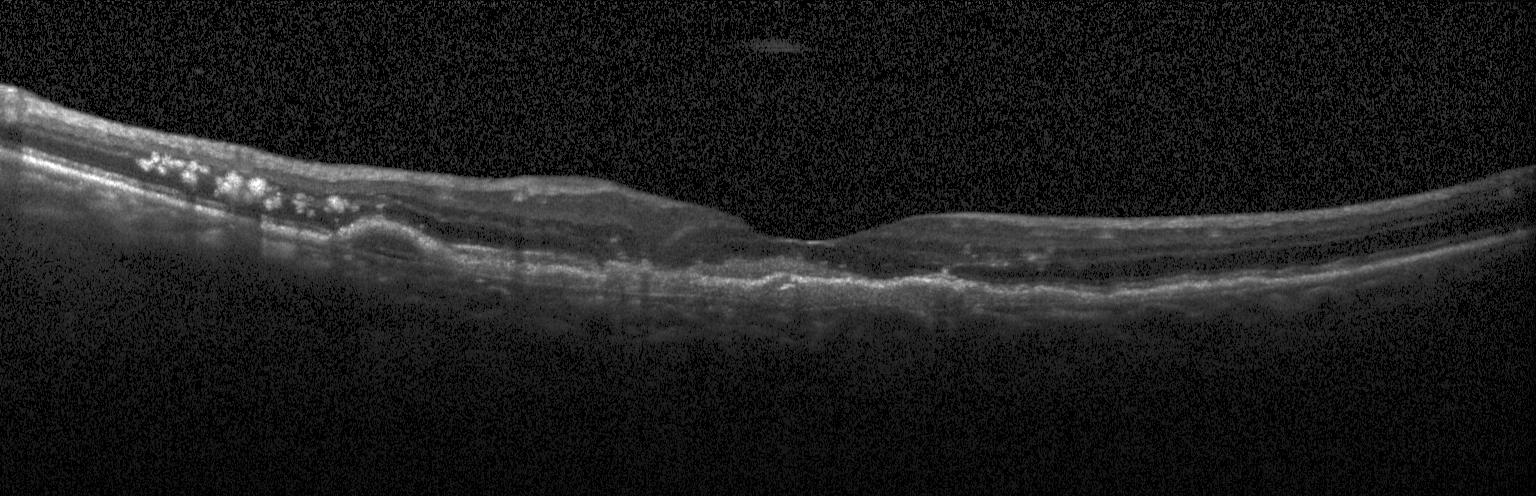 Impression: a choroidal neovascular membrane.